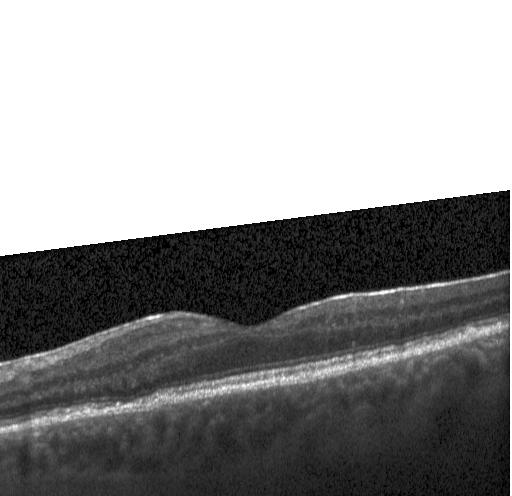
Heidelberg Spectralis OCT system, retinal OCT B-scan — Dx: neither choroidal neovascularization, diabetic macular edema, nor drusen.